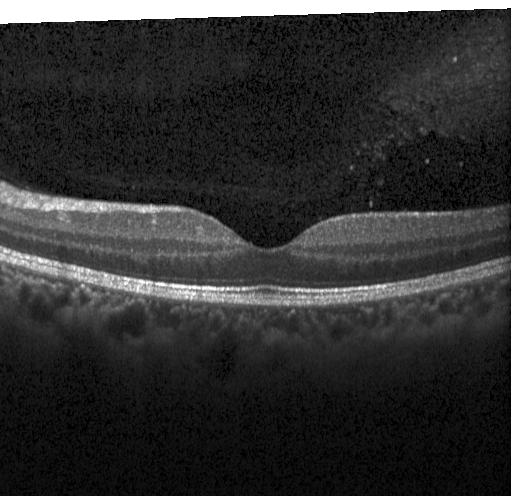
OCT B-scan — Diagnosis: no evidence of choroidal neovascularization, diabetic macular edema, or drusen.